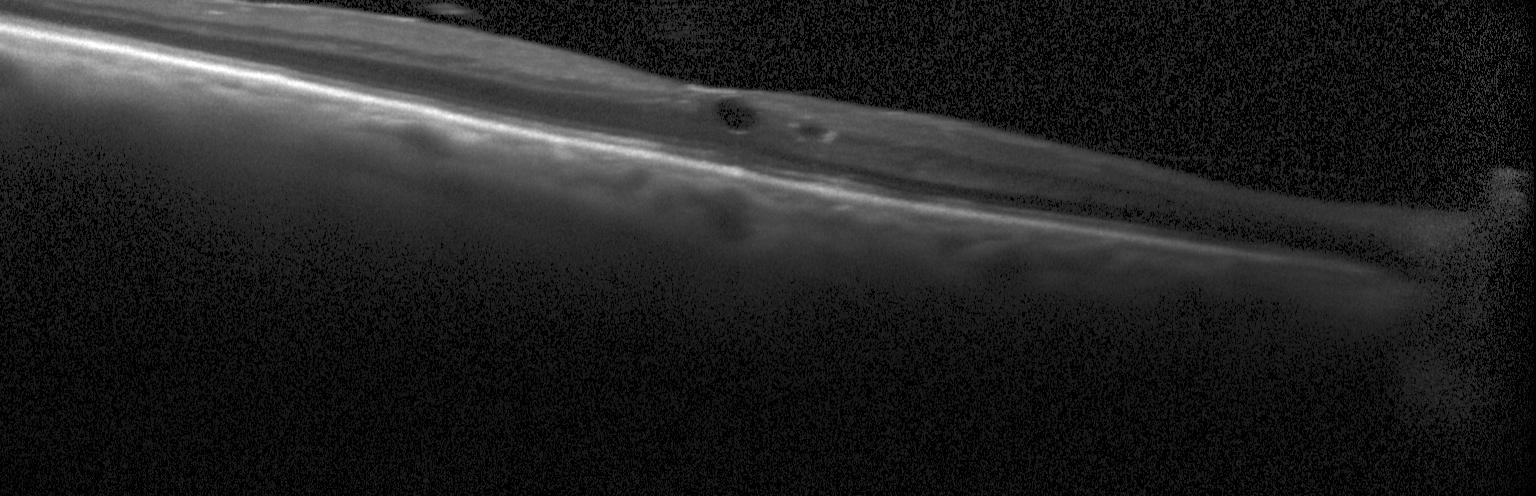 Optical coherence tomography scan.
Finding: diabetic macular edema.